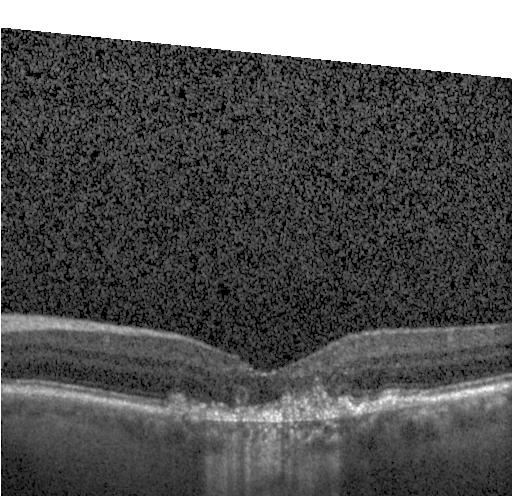 Acquired on a Heidelberg Spectralis; optical coherence tomography B-scan; spectral-domain OCT; macular scan — OCT finding: choroidal neovascularization.